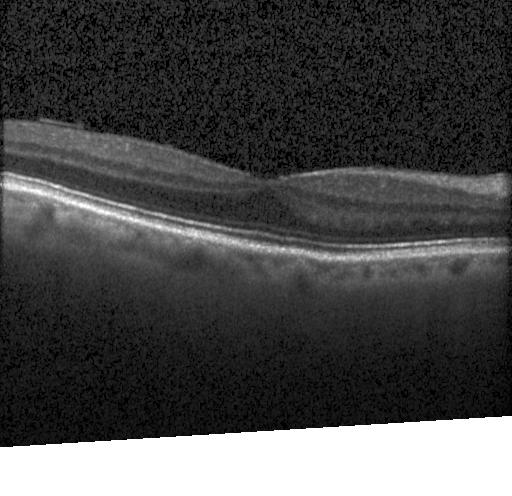 No choroidal neovascularization, diabetic macular edema, or drusen.